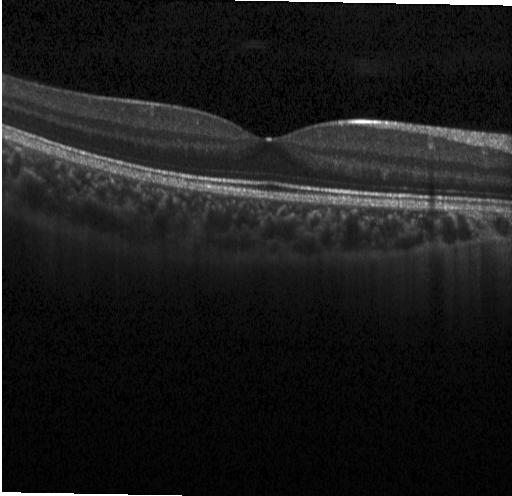 Macular scan; retinal OCT cross-section — This B-scan demonstrates neither CNV, DME, nor drusen.